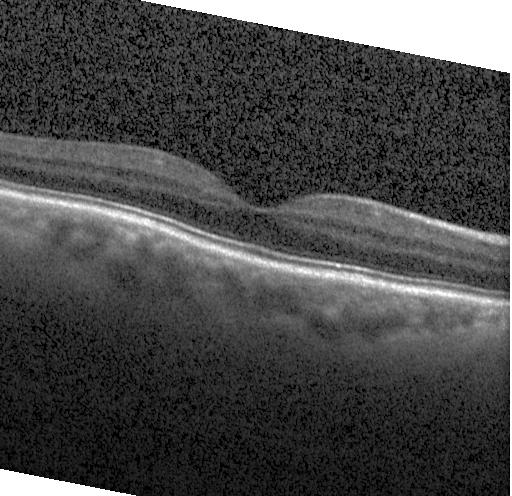 Finding: no evidence of choroidal neovascularization, diabetic macular edema, or drusen.